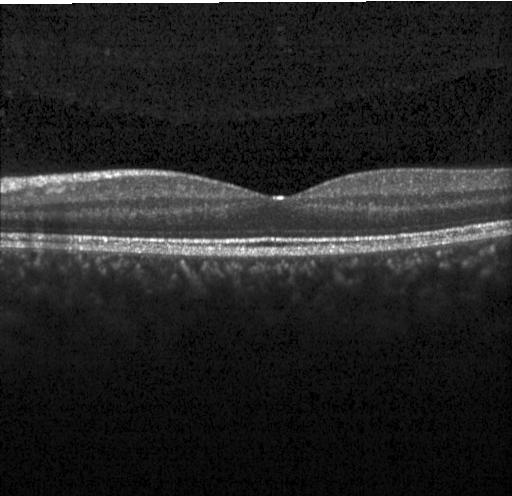
Retinal OCT B-scan, SD-OCT, centered on the fovea.
OCT finding: no choroidal neovascularization, no diabetic macular edema, and no drusen.